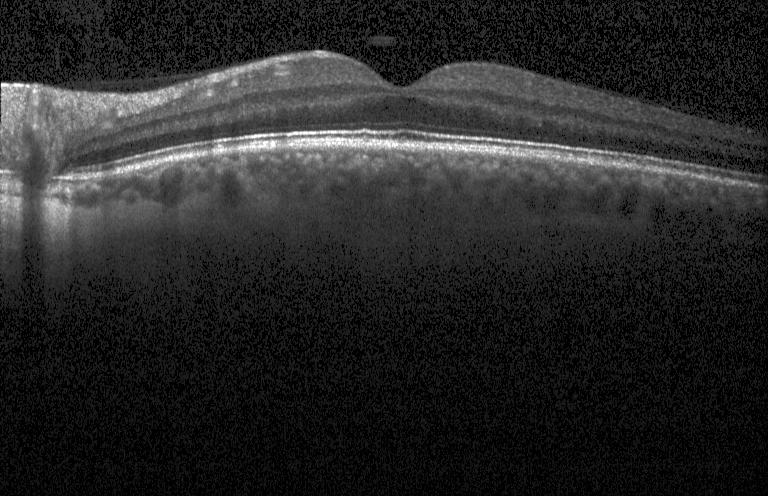
Instrument: Heidelberg Spectralis, spectral-domain optical coherence tomography, retinal OCT cross-section, through the macula. Finding: no evidence of choroidal neovascularization, diabetic macular edema, or drusen.